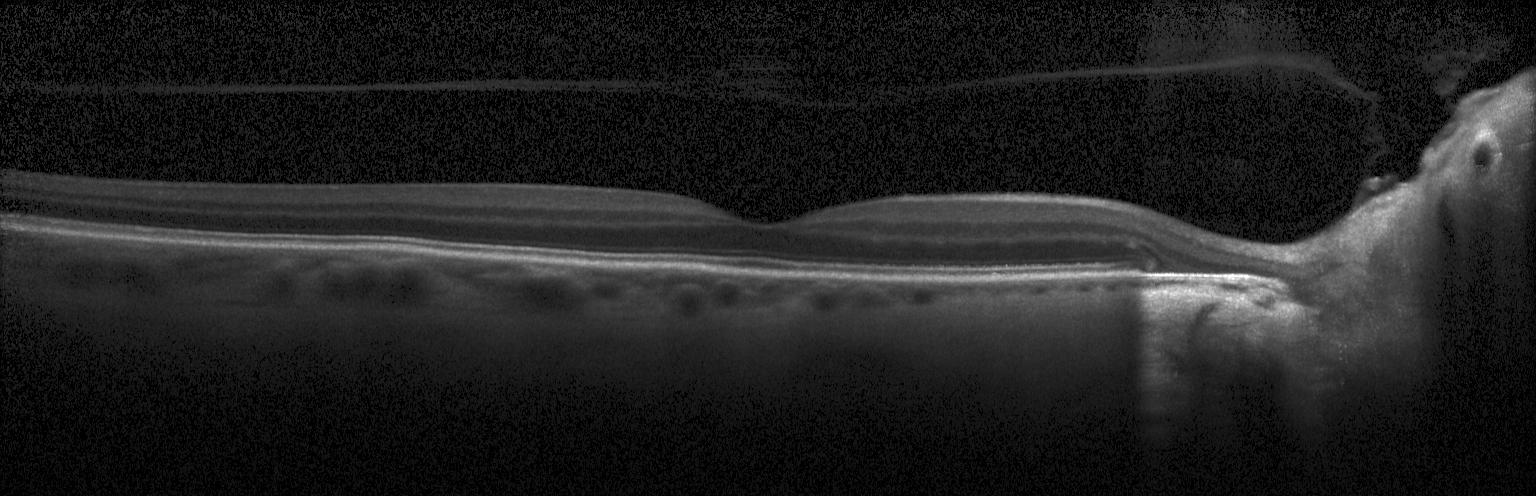

Retinal OCT cross-section. Finding: no choroidal neovascularization, diabetic macular edema, or drusen.